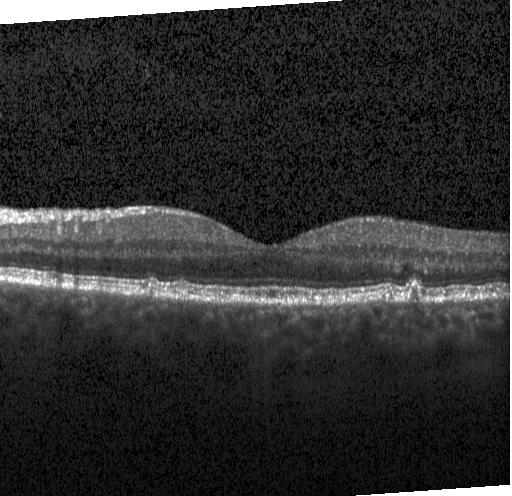

Drusen.